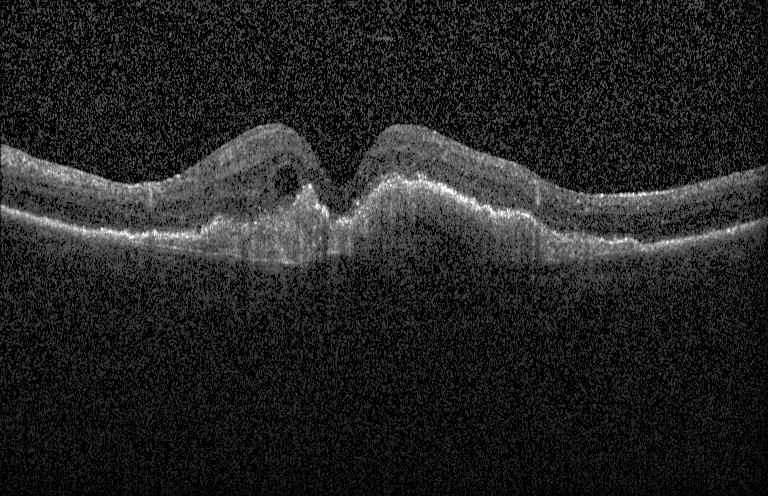
Impression: choroidal neovascularization.